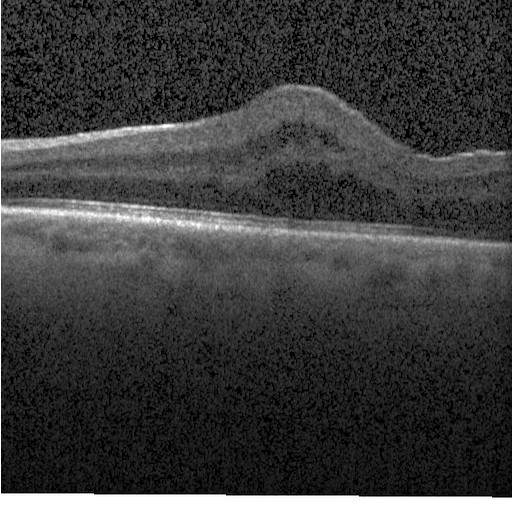

Horizontal scan through the fovea; acquired on a Heidelberg Spectralis; optical coherence tomography scan — Assessment: DME.